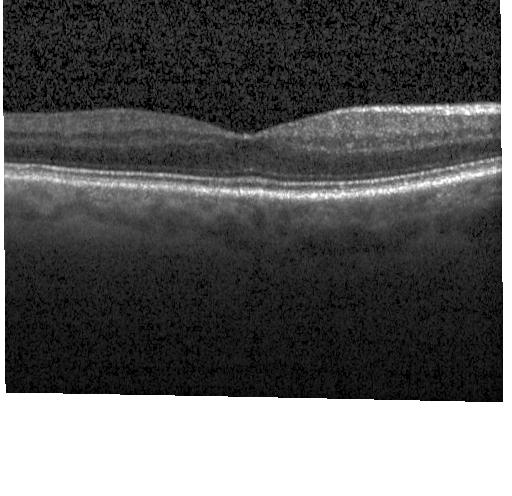 OCT line scan · spectral-domain OCT · Heidelberg Spectralis OCT system · macular scan — Diagnosis: no CNV, DME, or drusen.